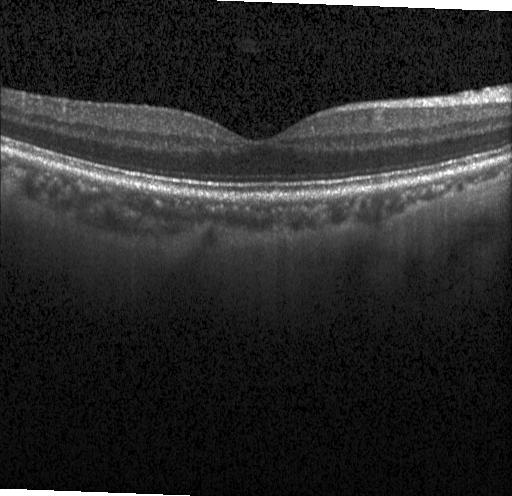 Optical coherence tomography B-scan; SD-OCT; macular scan
Dx: no choroidal neovascularization, no diabetic macular edema, and no drusen.